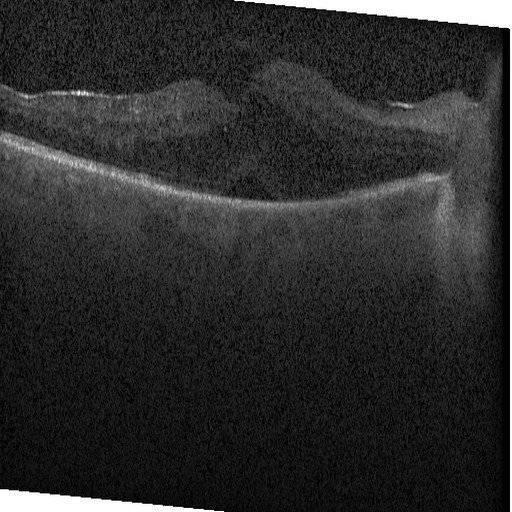
Centered on the fovea. SD-OCT. Heidelberg Spectralis OCT system. Optical coherence tomography scan. This B-scan demonstrates diabetic macular edema.